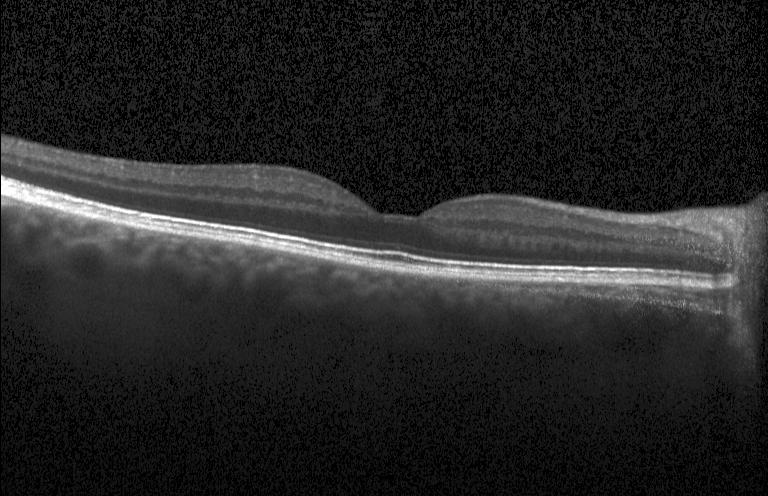 Retinal OCT cross-section showing no evidence of choroidal neovascularization, diabetic macular edema, or drusen.